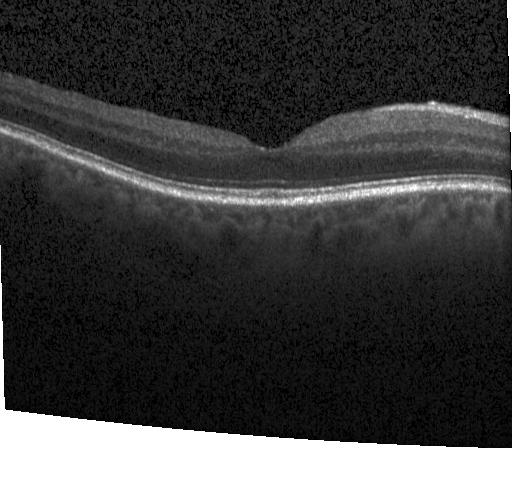

SD-OCT · optical coherence tomography B-scan · instrument: Heidelberg Spectralis.
OCT finding: no choroidal neovascularization, diabetic macular edema, or drusen.